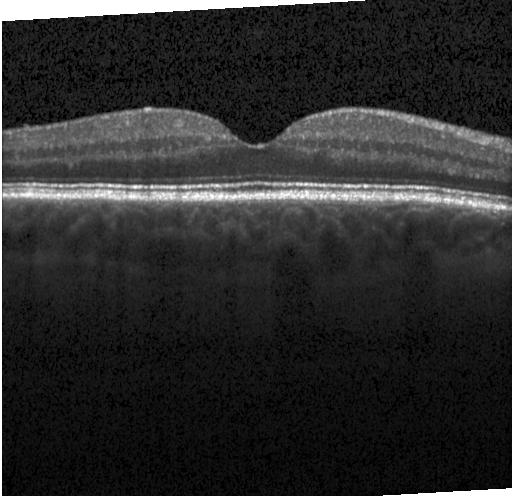

Centered on the fovea. Optical coherence tomography B-scan. Acquired on a Heidelberg Spectralis — Impression: neither CNV, DME, nor drusen.